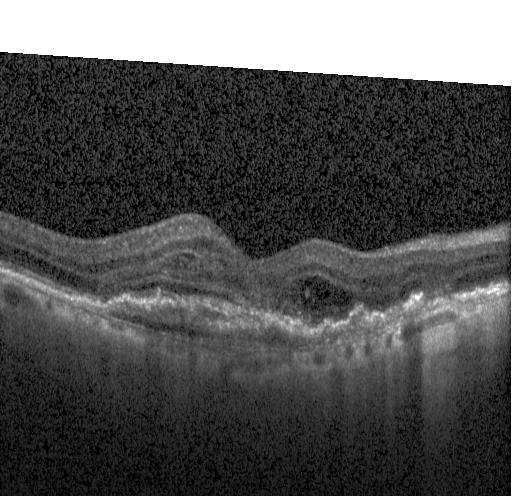
Spectral-domain OCT, optical coherence tomography B-scan, acquired on a Heidelberg Spectralis, fovea-centered — Impression: CNV.